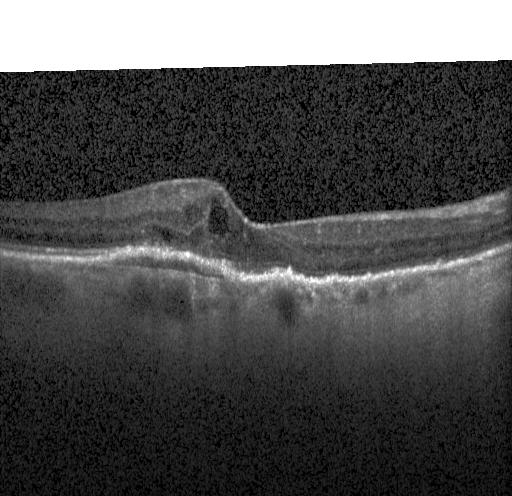 Optical coherence tomography B-scan. Dx: choroidal neovascularization (CNV).